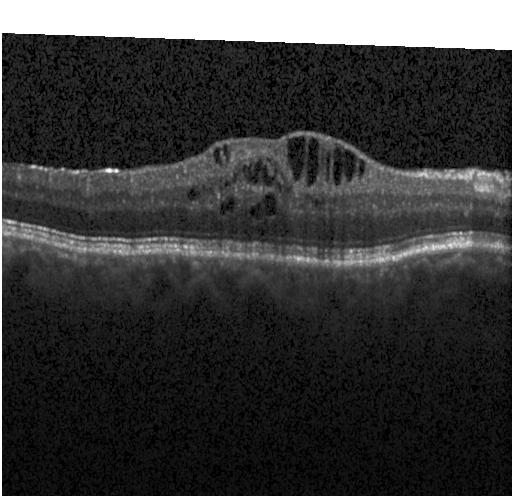 Retinal OCT B-scan
Diagnosis: diabetic macular edema (DME).